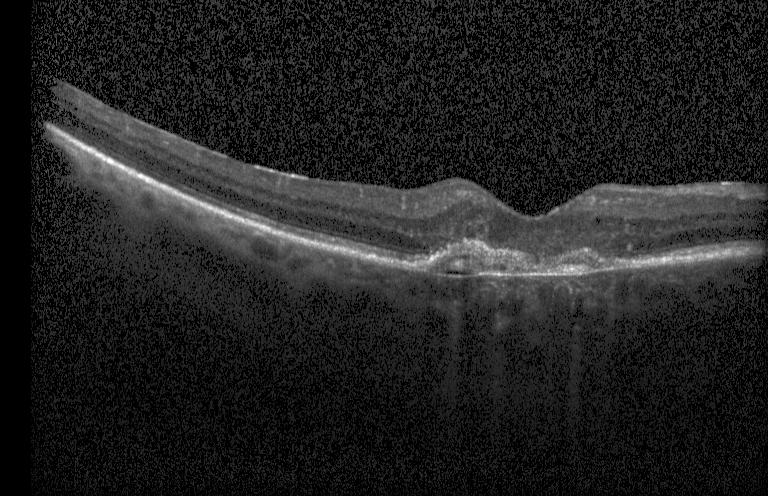 Impression: a choroidal neovascular membrane.